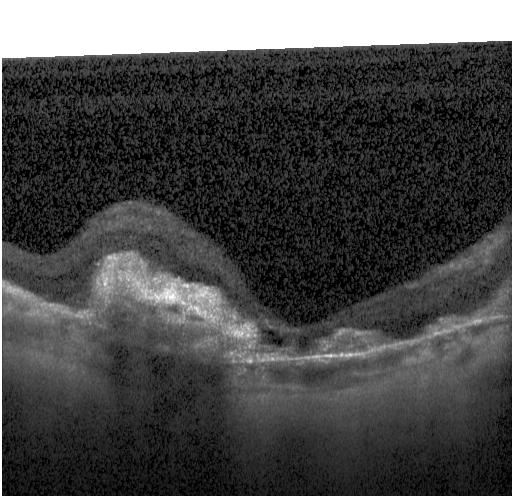 Dx: a choroidal neovascular membrane.